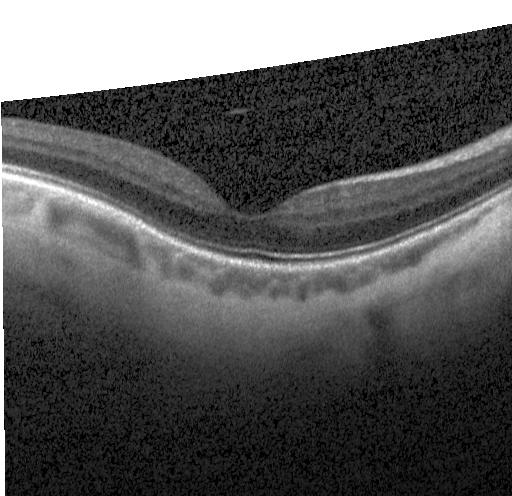

Fovea-centered · OCT line scan · Heidelberg Spectralis OCT system · spectral-domain OCT.
Finding: neither choroidal neovascularization, diabetic macular edema, nor drusen.